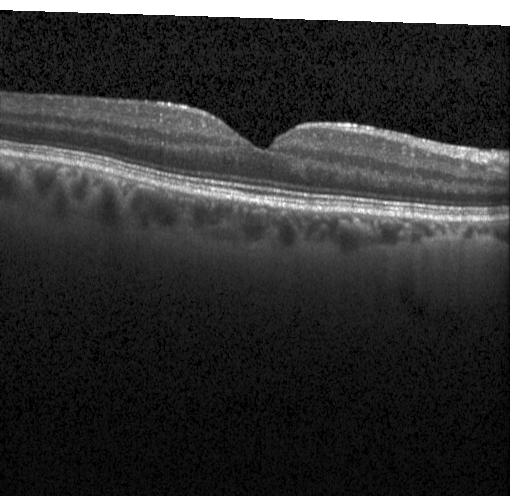 Diagnosis: no CNV, no DME, and no drusen.